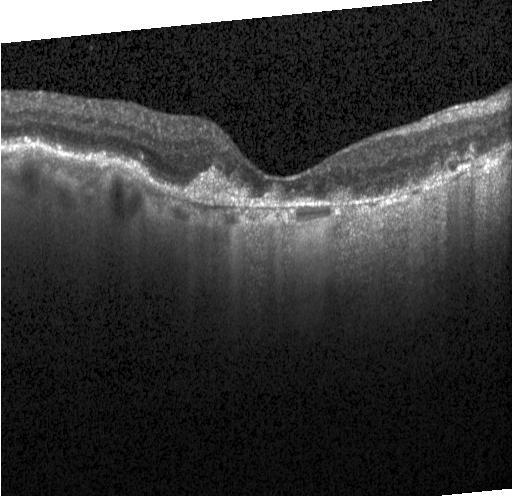 Instrument: Heidelberg Spectralis · OCT B-scan. Assessment: choroidal neovascularization.